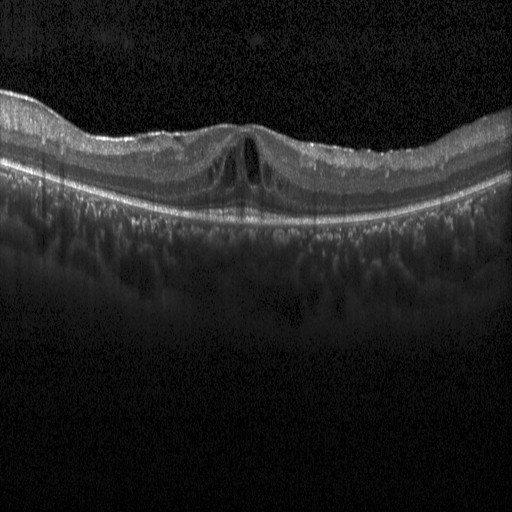

Acquired on a Heidelberg Spectralis · OCT line scan — The scan shows diabetic macular edema (DME).